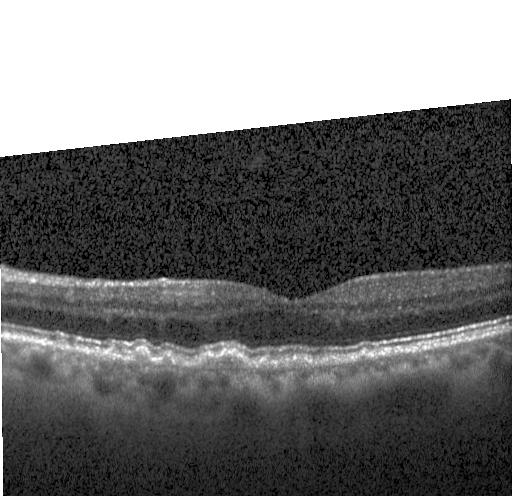
Finding: multiple drusen.